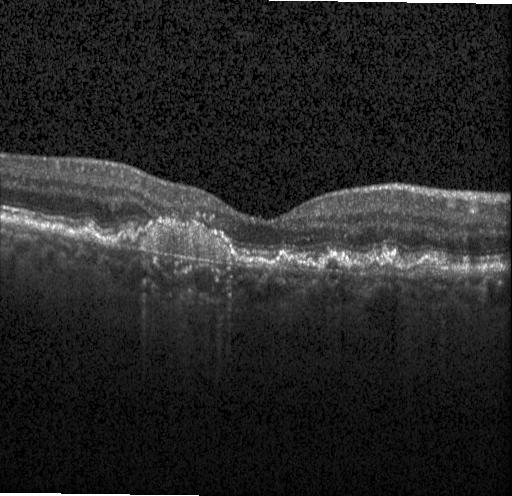 Spectral-domain optical coherence tomography, instrument: Heidelberg Spectralis, OCT line scan, through the macula. The scan shows CNV.